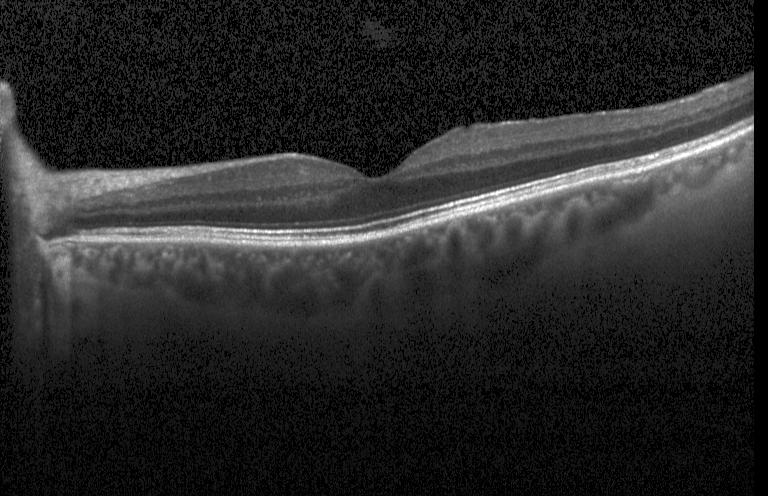

Spectral-domain optical coherence tomography, retinal OCT cross-section — Assessment: no evidence of choroidal neovascularization, diabetic macular edema, or drusen.